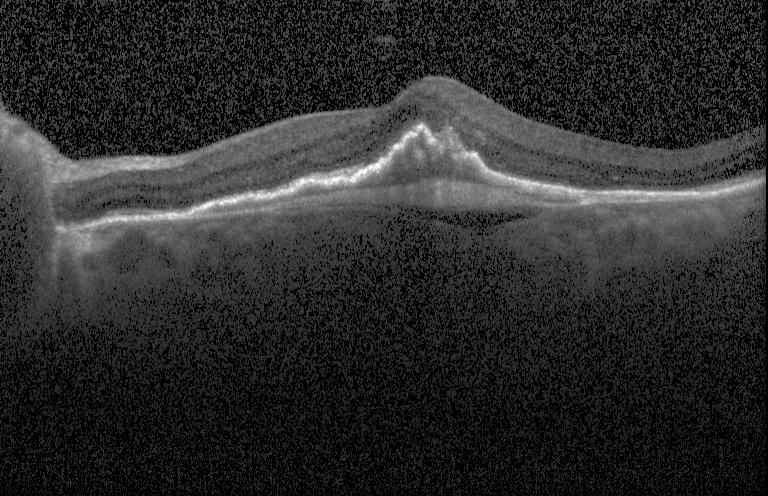
SD-OCT · optical coherence tomography B-scan. Finding: CNV.